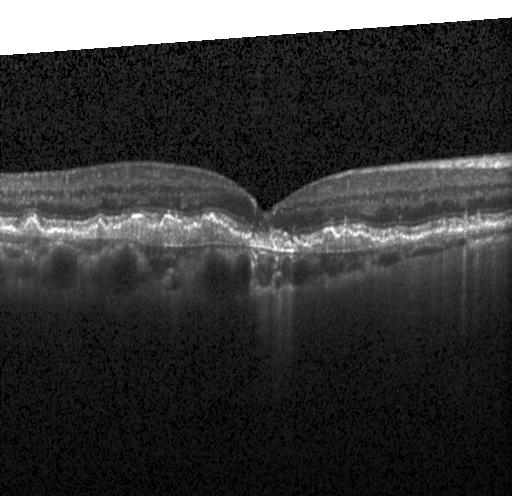
Diagnosis: choroidal neovascularization.